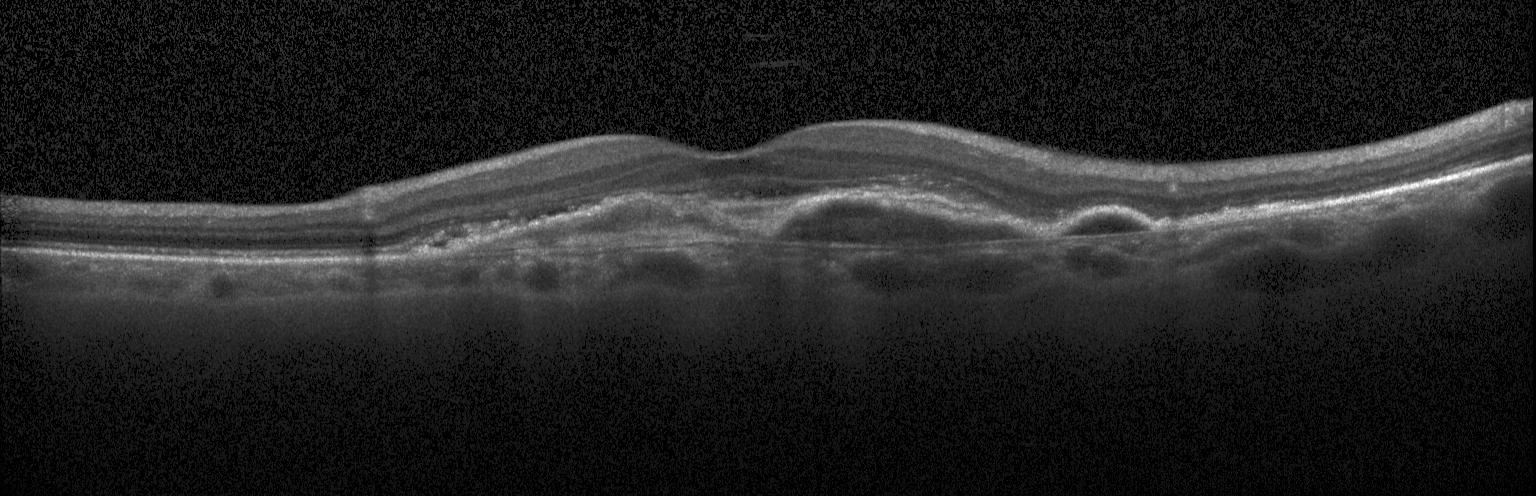
Optical coherence tomography B-scan.
Impression: CNV.